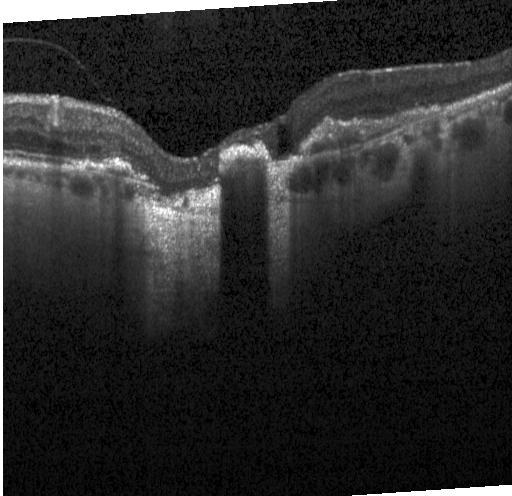
Retinal OCT B-scan. CNV.